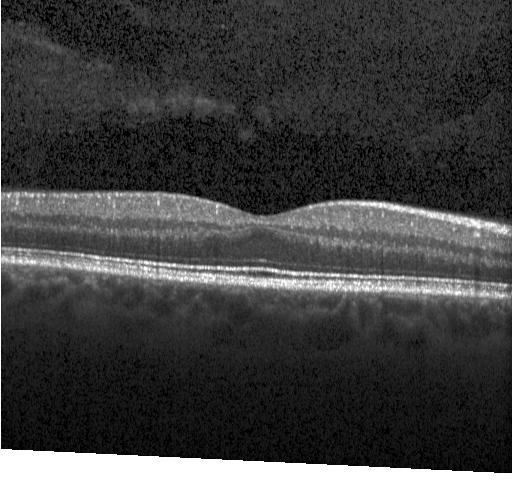
Horizontal scan through the fovea · spectral-domain OCT · Heidelberg Spectralis OCT system · optical coherence tomography scan. Assessment: no evidence of choroidal neovascularization, diabetic macular edema, or drusen.